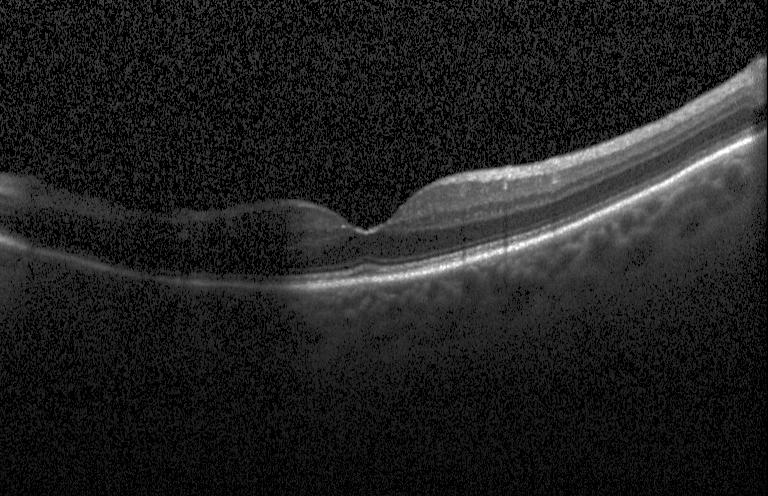

Assessment: no choroidal neovascularization, diabetic macular edema, or drusen.